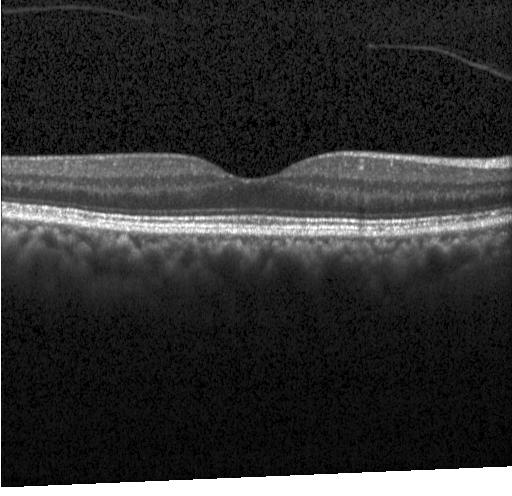 Finding: no evidence of choroidal neovascularization, diabetic macular edema, or drusen.